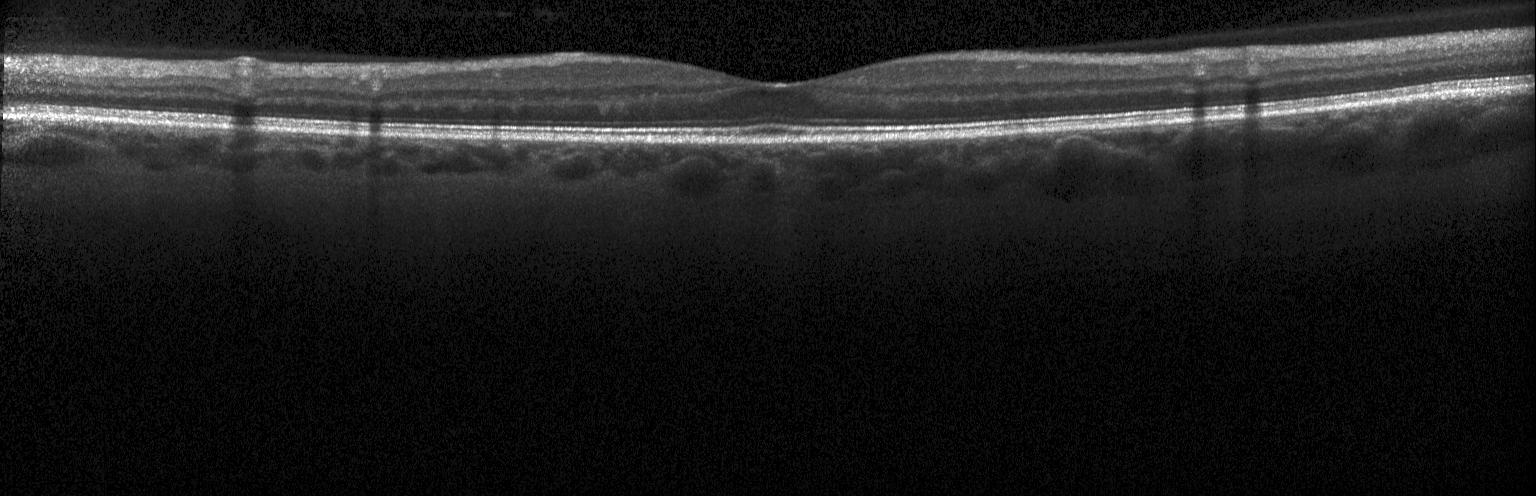

Retinal OCT B-scan. Heidelberg Spectralis OCT system — Dx: no evidence of CNV, DME, or drusen.